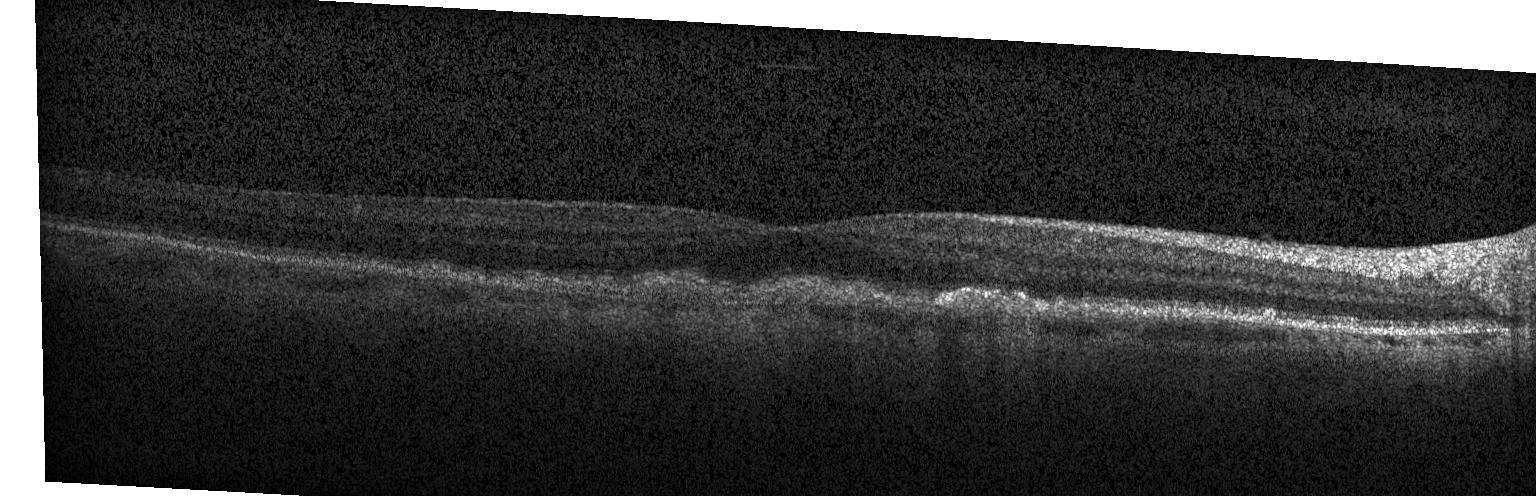

OCT scan showing a choroidal neovascular membrane.